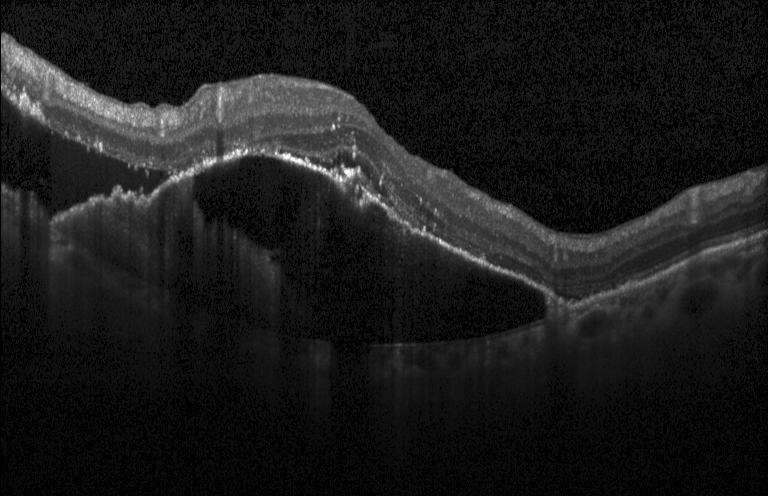
Retinal OCT cross-section. The scan shows choroidal neovascularization (CNV).